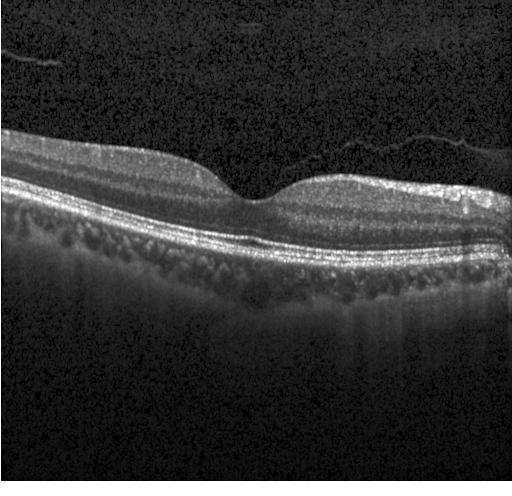 Optical coherence tomography B-scan — This B-scan demonstrates neither choroidal neovascularization, diabetic macular edema, nor drusen.